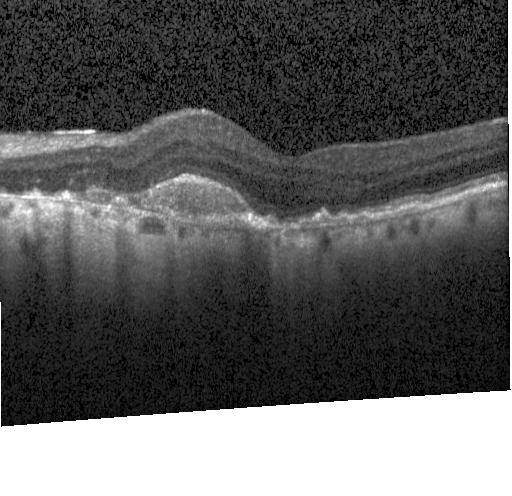

Optical coherence tomography B-scan.
Diagnosis: CNV.